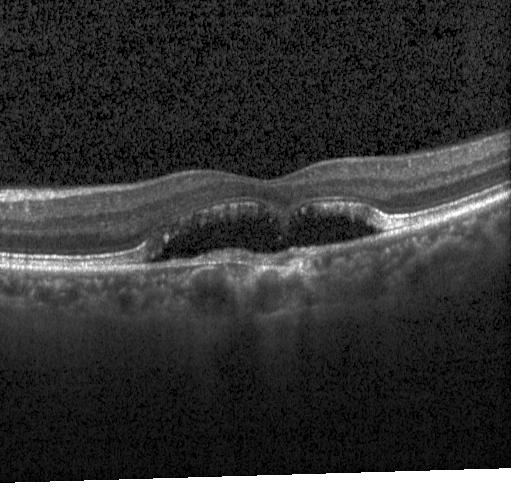
Impression: choroidal neovascularization.